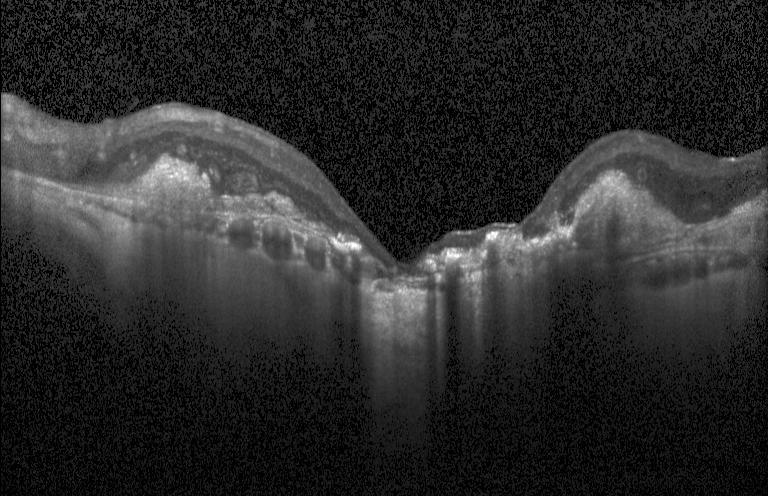

Through the macula, optical coherence tomography scan, instrument: Heidelberg Spectralis
Choroidal neovascularization (CNV).